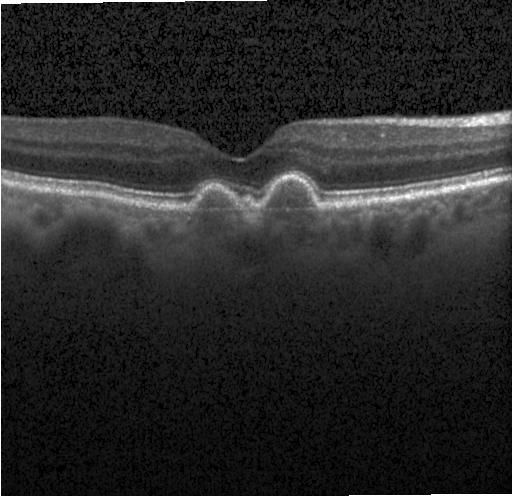
Retinal OCT cross-section showing drusen.